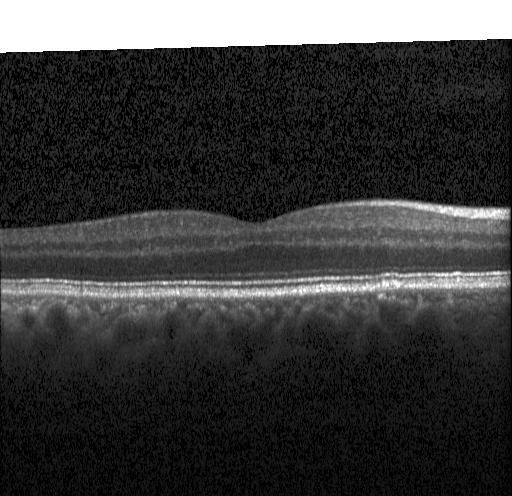
Diagnosis: neither choroidal neovascularization, diabetic macular edema, nor drusen.